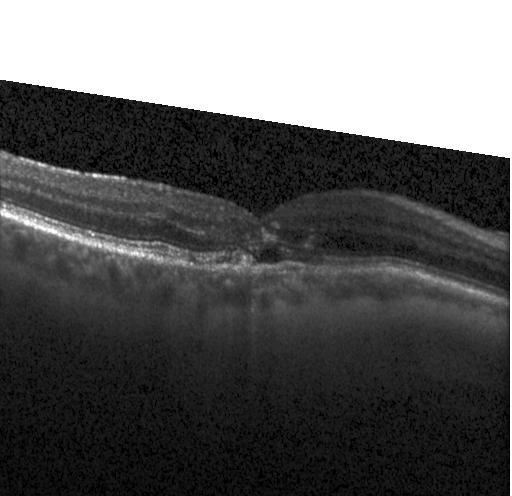

Heidelberg Spectralis. Retinal OCT cross-section
Diagnosis: CNV.